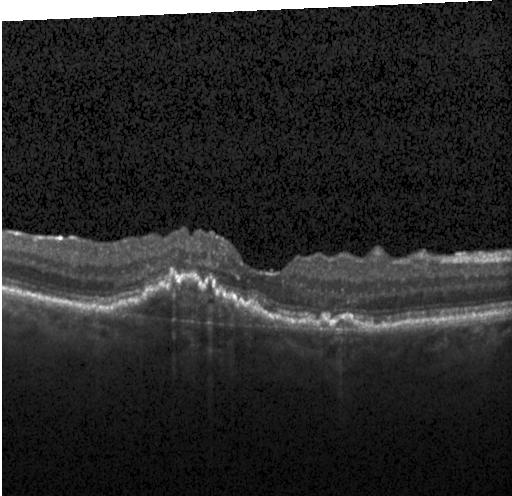

Heidelberg Spectralis · optical coherence tomography B-scan
OCT finding: a choroidal neovascular membrane.